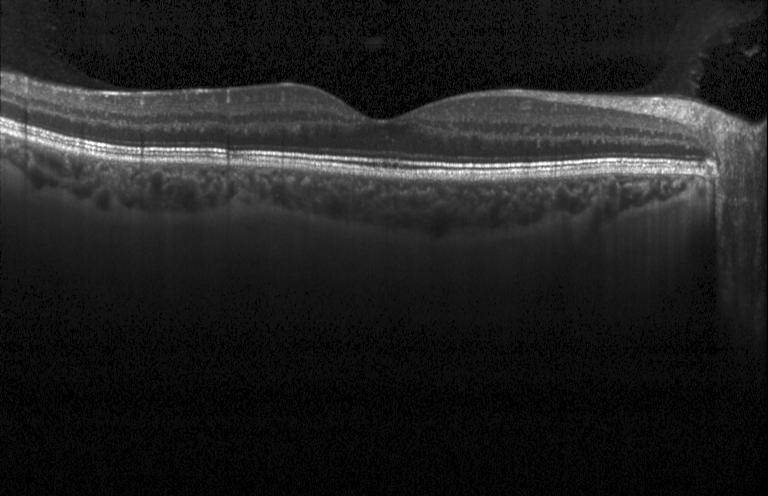

Macular OCT: no evidence of choroidal neovascularization, diabetic macular edema, or drusen.